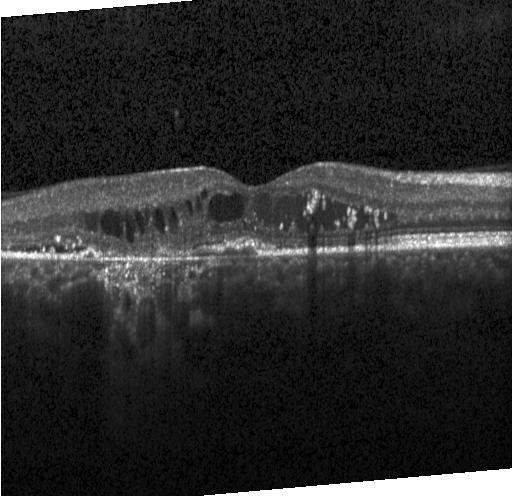 OCT scan showing CNV.